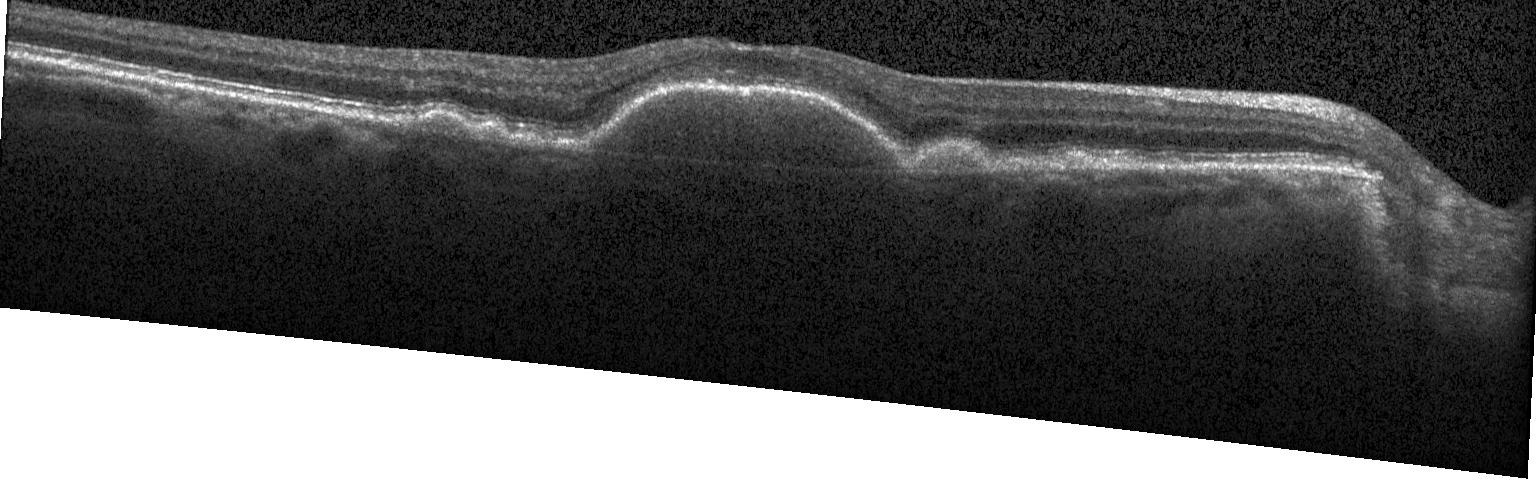 This B-scan demonstrates choroidal neovascularization (CNV).